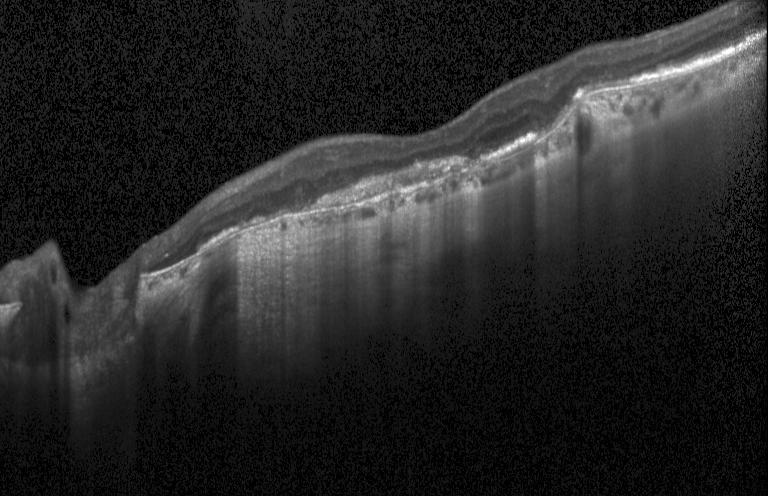

A choroidal neovascular membrane.